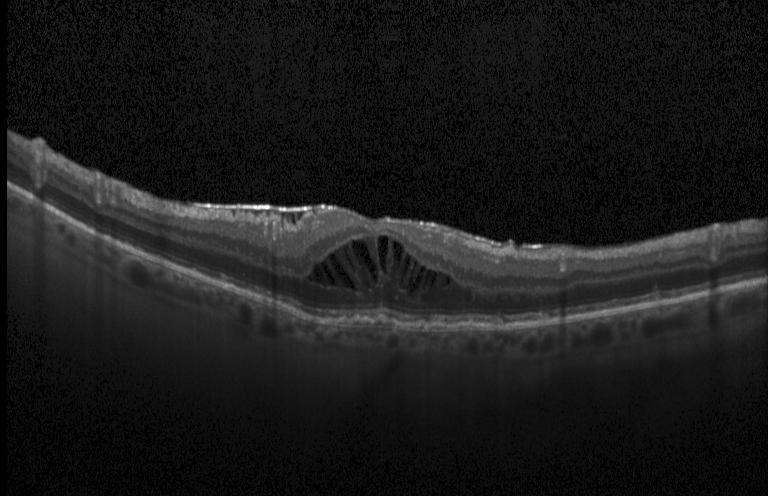

Horizontal scan through the fovea, Heidelberg Spectralis, spectral-domain OCT, OCT line scan — Macular OCT: diabetic macular edema (DME).